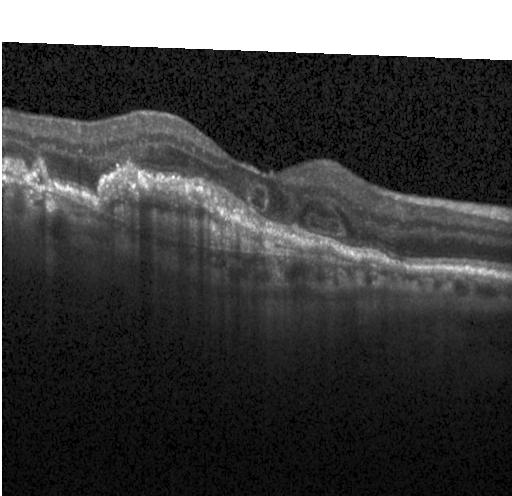
Dx: choroidal neovascularization.